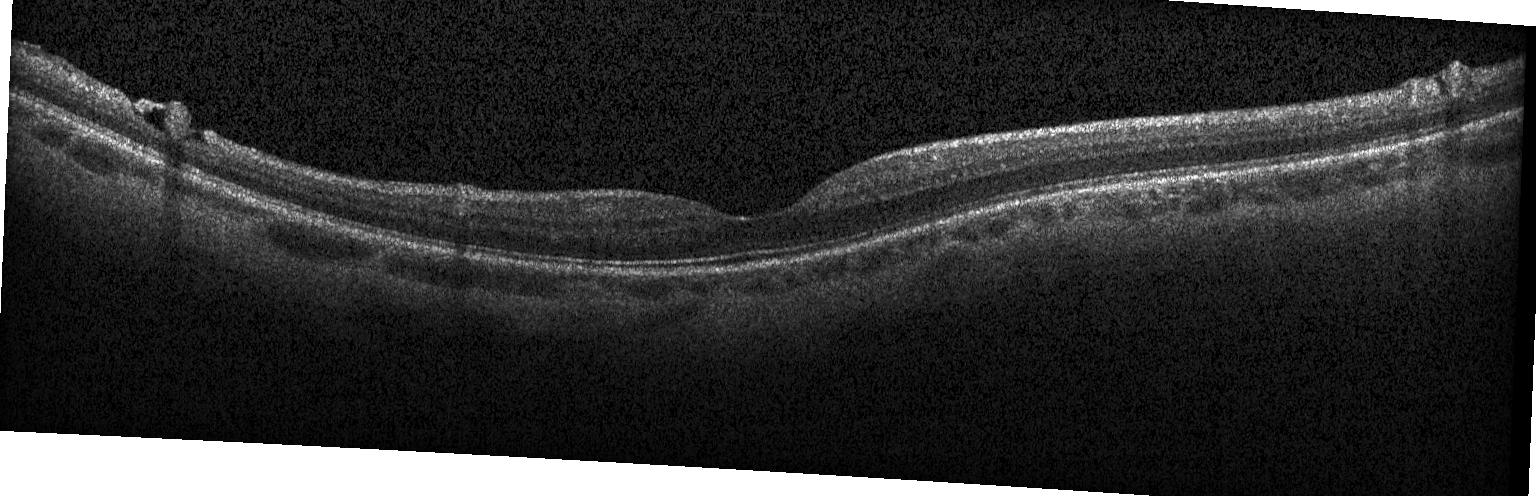
OCT scan showing neither choroidal neovascularization, diabetic macular edema, nor drusen.